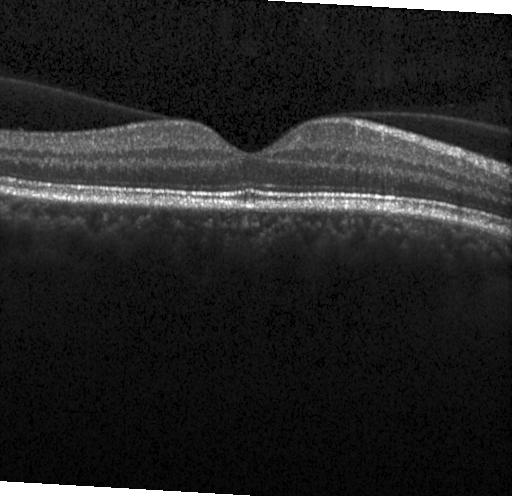
Optical coherence tomography scan, spectral-domain OCT.
Neither choroidal neovascularization, diabetic macular edema, nor drusen.